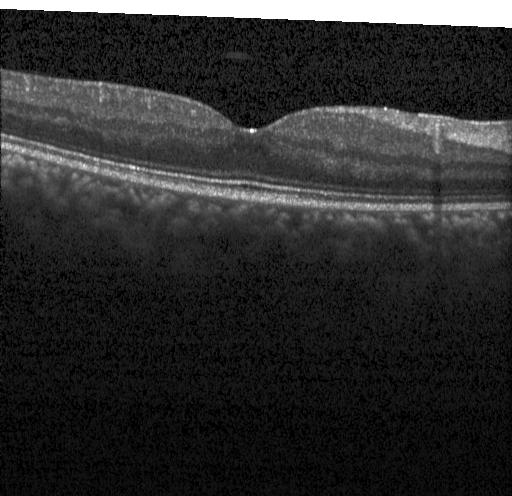

Optical coherence tomography scan, fovea-centered, spectral-domain optical coherence tomography, acquired on a Heidelberg Spectralis
Neither CNV, DME, nor drusen.